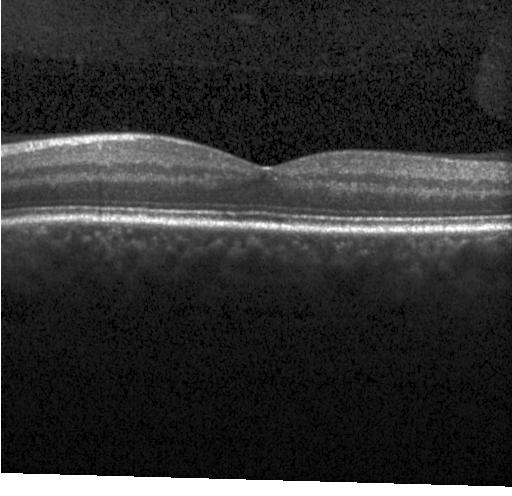

OCT line scan. Heidelberg Spectralis. SD-OCT. Diagnosis: no CNV, no DME, and no drusen.